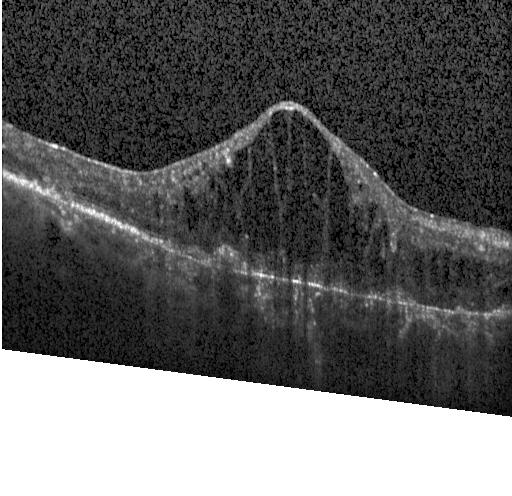 Diagnosis: choroidal neovascularization.